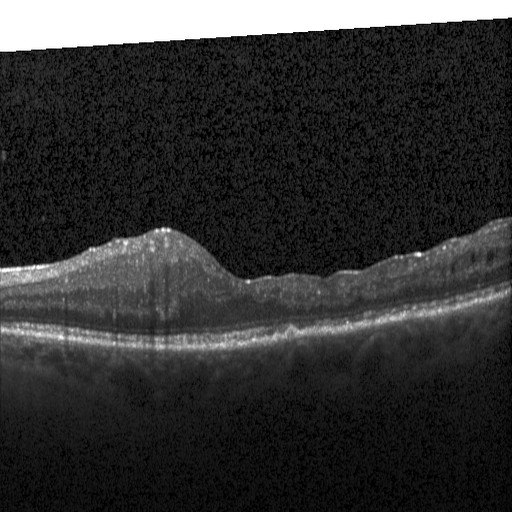 Optical coherence tomography B-scan — Diagnosis: DME.